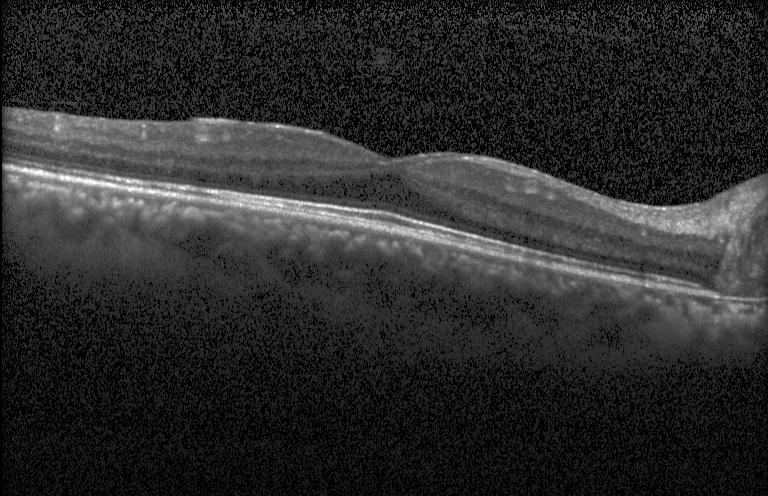 The scan shows no choroidal neovascularization, no diabetic macular edema, and no drusen.